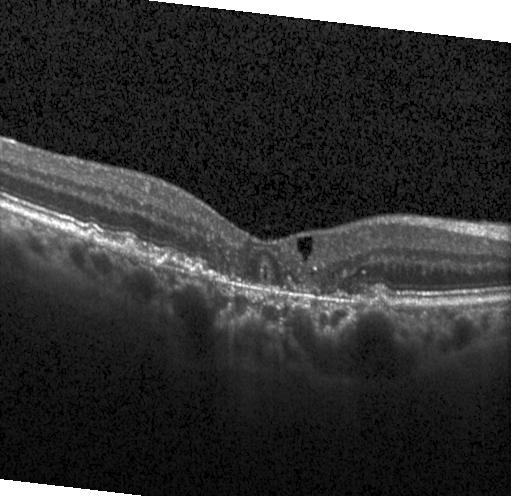 Macular OCT demonstrating CNV.